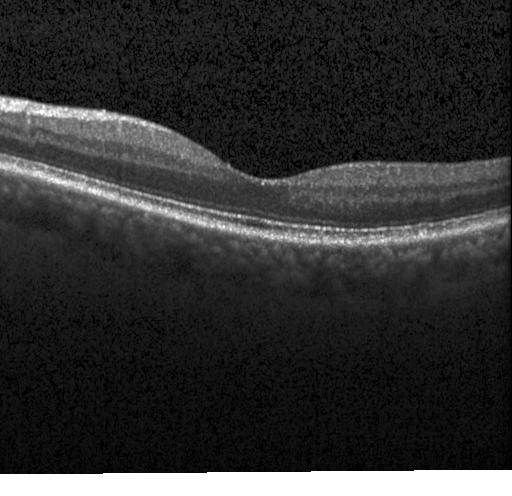
Macular OCT: neither CNV, DME, nor drusen.